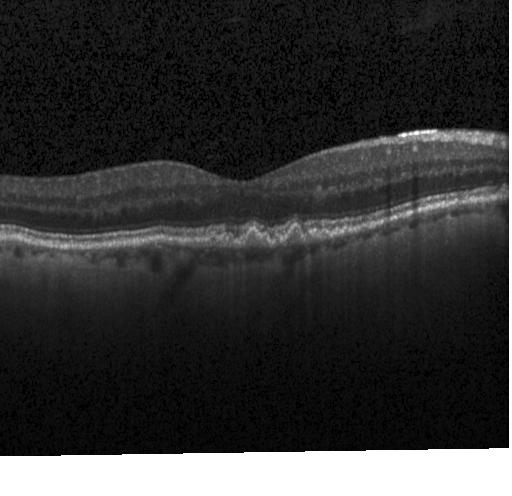
SD-OCT; centered on the fovea; OCT B-scan. Finding: multiple drusen.